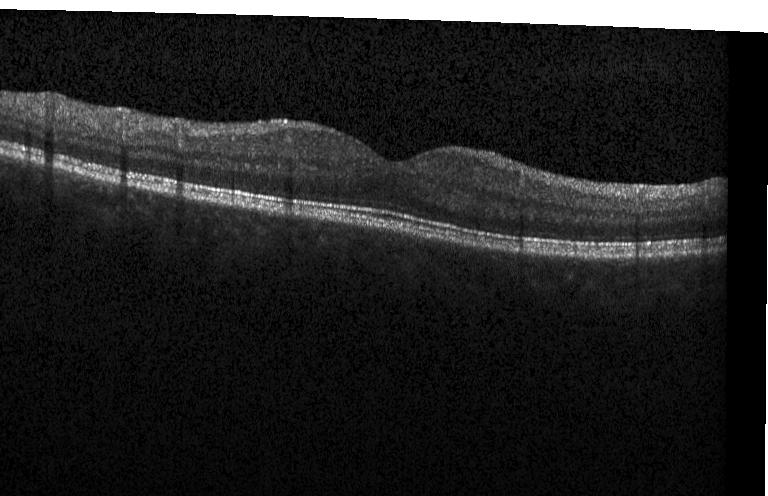
OCT line scan. Spectral-domain optical coherence tomography. Finding: neither choroidal neovascularization, diabetic macular edema, nor drusen.